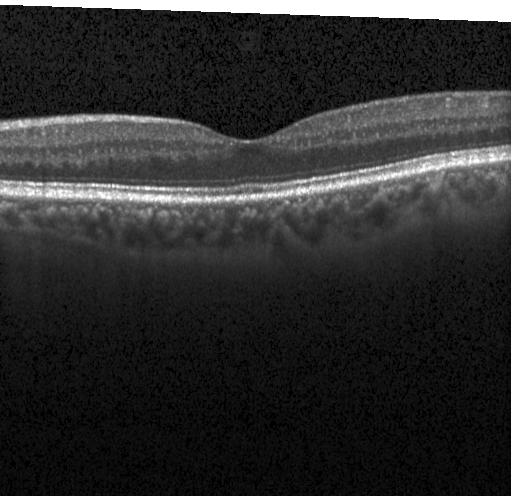 Fovea-centered; OCT B-scan; SD-OCT
Impression: no evidence of choroidal neovascularization, diabetic macular edema, or drusen.